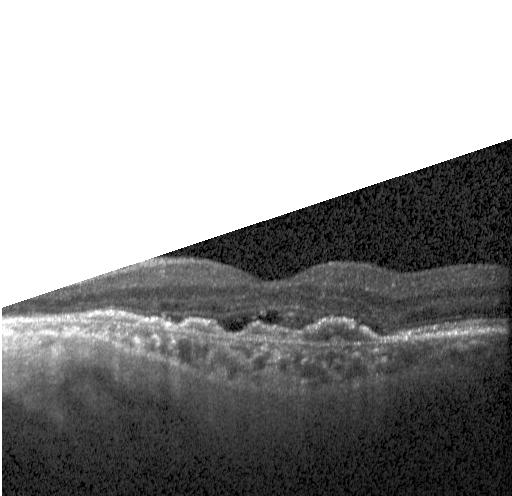 Finding: a choroidal neovascular membrane.